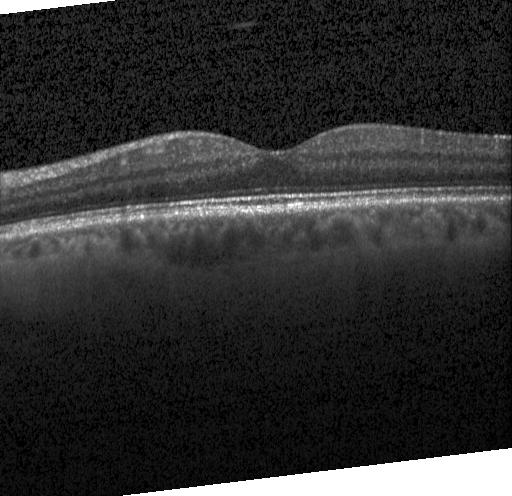 SD-OCT. Retinal OCT cross-section. Heidelberg Spectralis.
Macular OCT: neither CNV, DME, nor drusen.